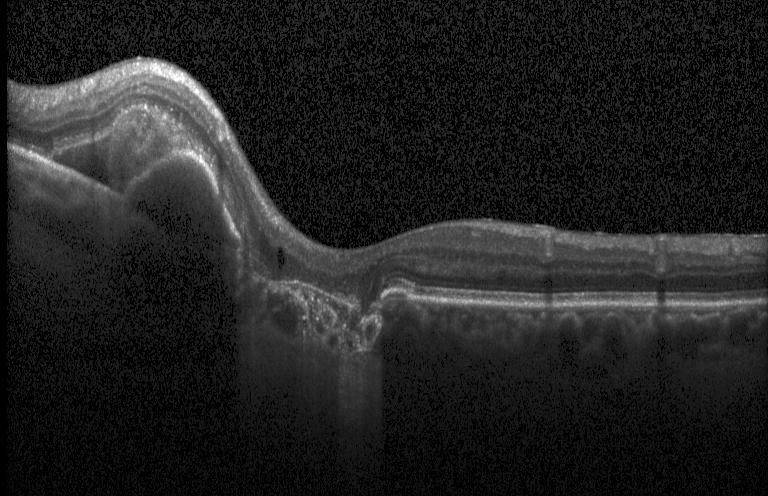
Instrument: Heidelberg Spectralis; retinal OCT cross-section — This B-scan demonstrates choroidal neovascularization (CNV).